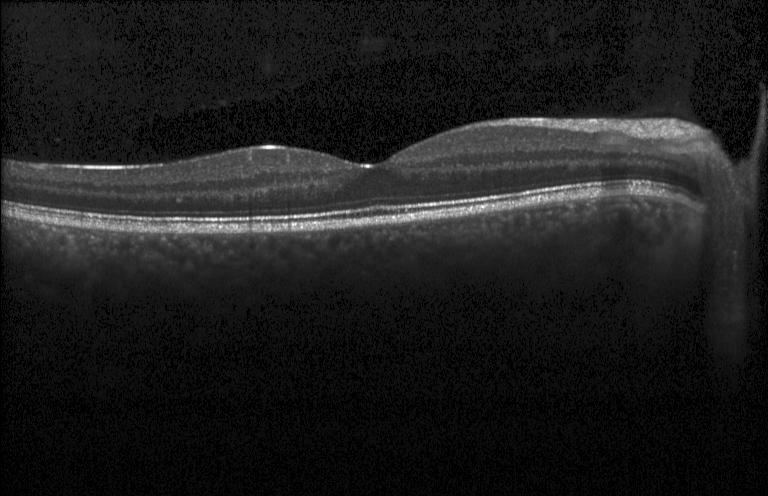
Macular scan; optical coherence tomography B-scan.
Assessment: no CNV, no DME, and no drusen.